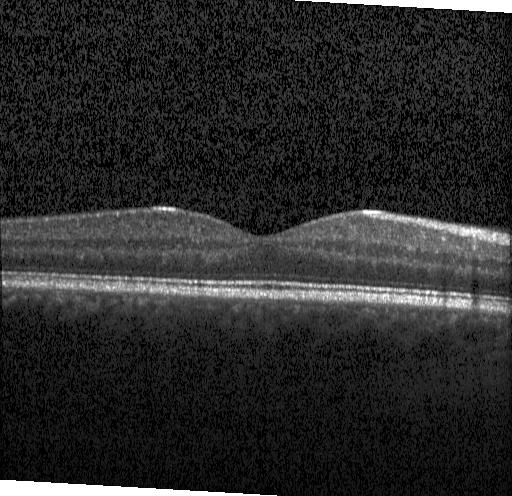
This B-scan demonstrates neither choroidal neovascularization, diabetic macular edema, nor drusen.